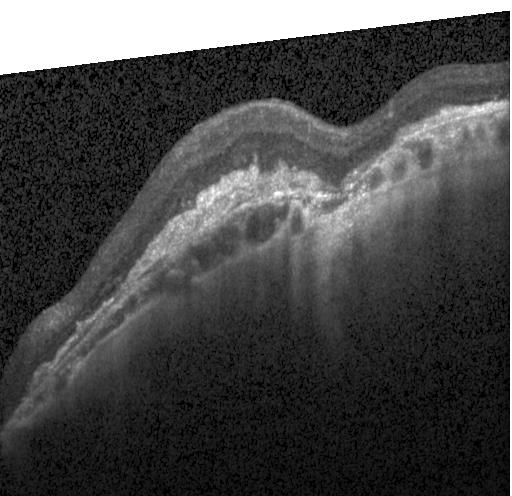
Macular scan, retinal OCT cross-section, Heidelberg Spectralis.
OCT finding: choroidal neovascularization.